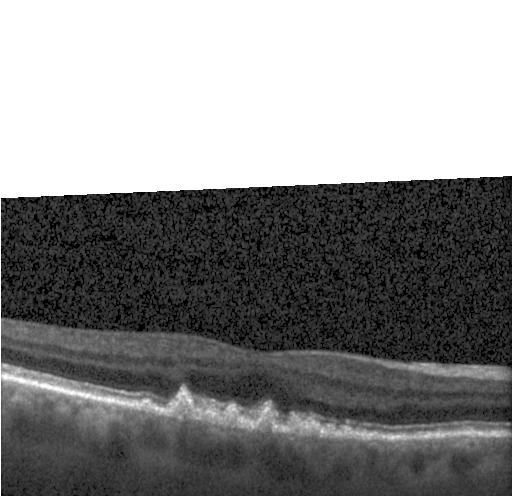
Optical coherence tomography scan · centered on the fovea · spectral-domain optical coherence tomography · Heidelberg Spectralis — Impression: sub-RPE drusenoid deposits.